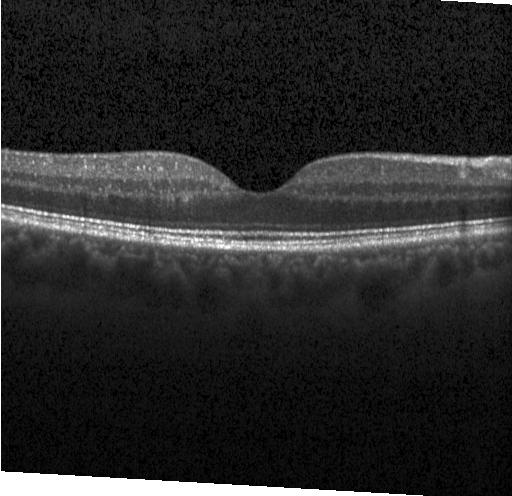

Neither CNV, DME, nor drusen.